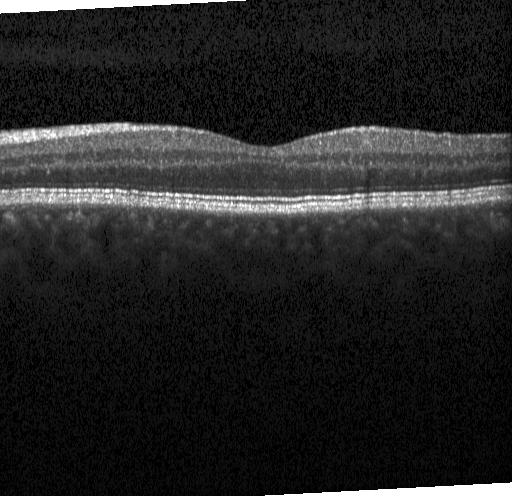 Impression: neither choroidal neovascularization, diabetic macular edema, nor drusen.